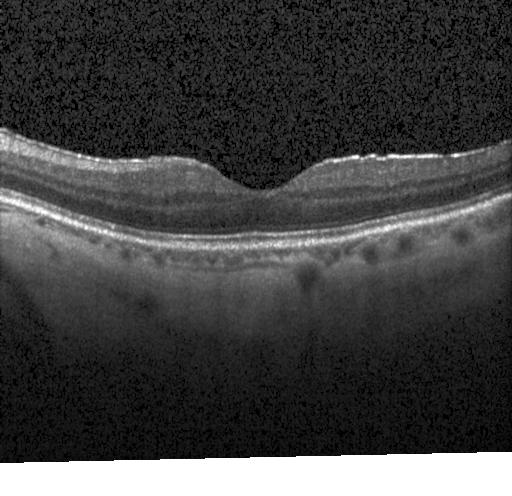 Retinal OCT B-scan; horizontal scan through the fovea. Impression: no evidence of choroidal neovascularization, diabetic macular edema, or drusen.